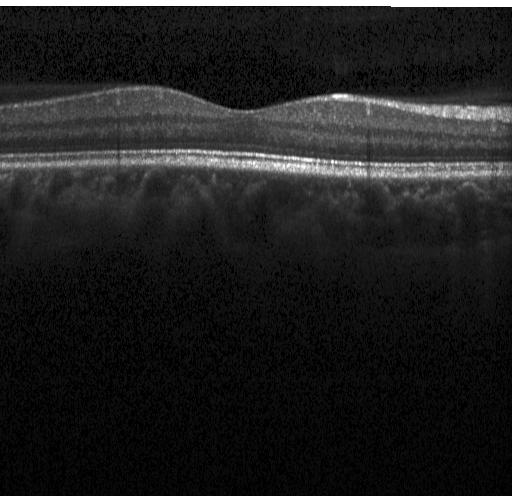 Instrument: Heidelberg Spectralis. Retinal OCT B-scan
Finding: neither choroidal neovascularization, diabetic macular edema, nor drusen.